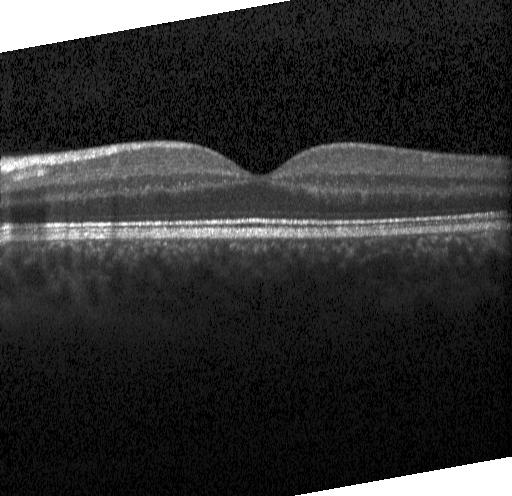
Retinal OCT cross-section — Assessment: neither CNV, DME, nor drusen.